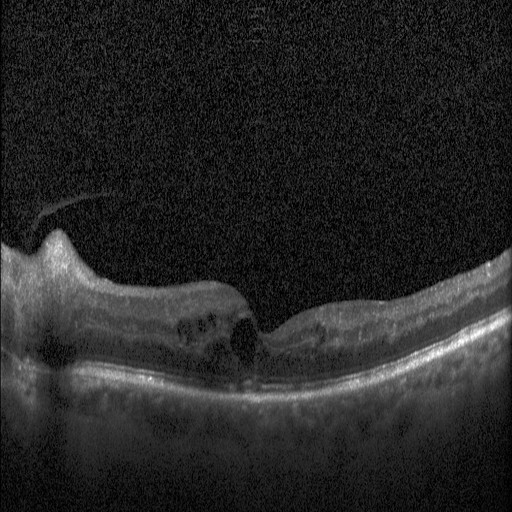 Heidelberg Spectralis, SD-OCT, retinal OCT B-scan.
Impression: diabetic macular edema.